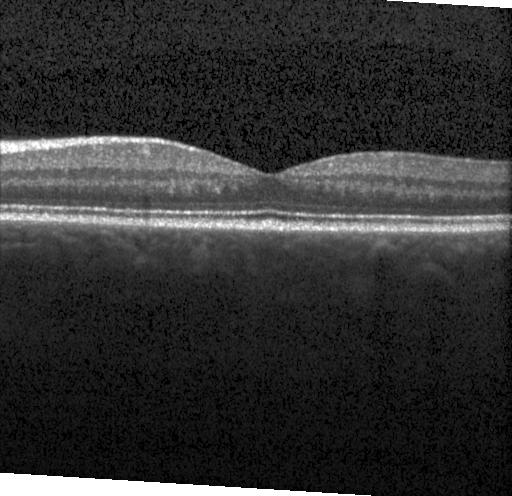 OCT B-scan, SD-OCT, Heidelberg Spectralis OCT system.
Dx: no evidence of choroidal neovascularization, diabetic macular edema, or drusen.